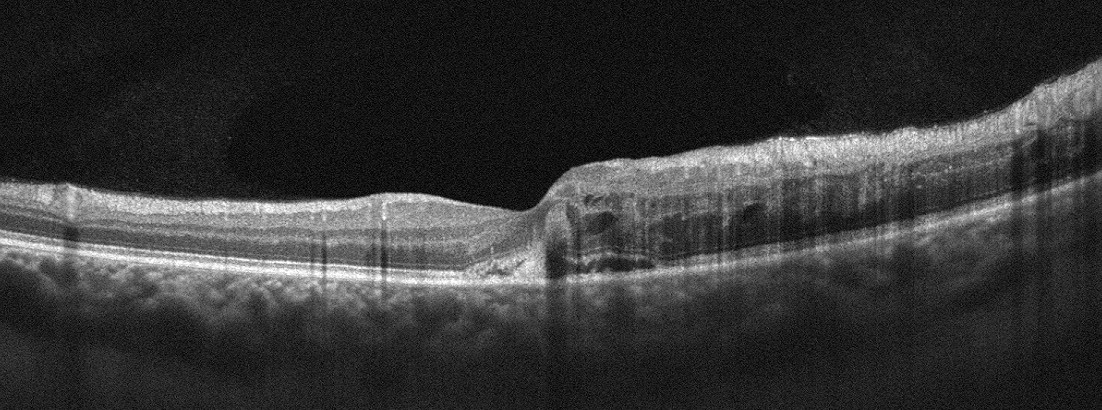 OCT B-scan
OCT finding: retinal vein occlusion (RVO).